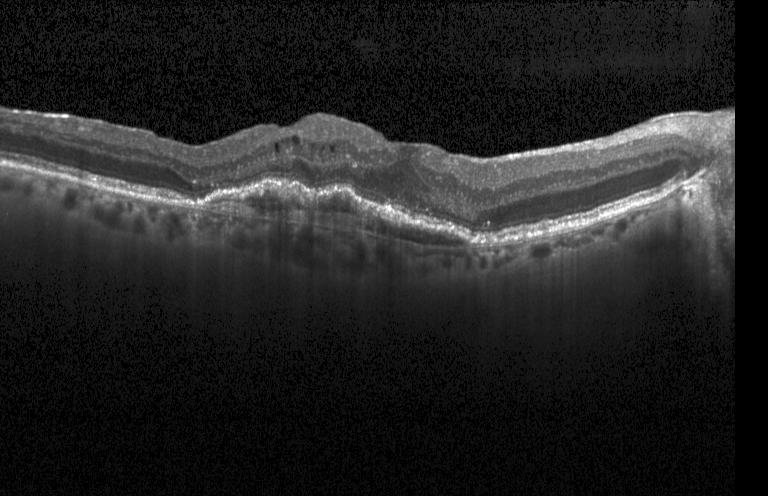

Choroidal neovascularization.